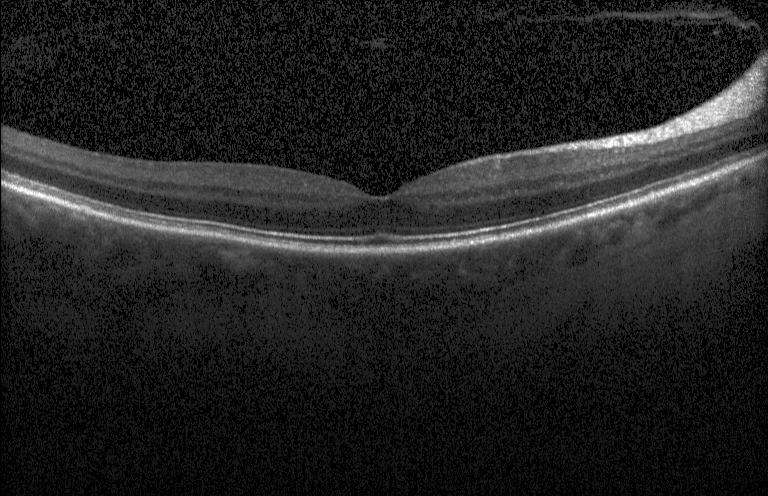 Dx: no choroidal neovascularization, diabetic macular edema, or drusen.